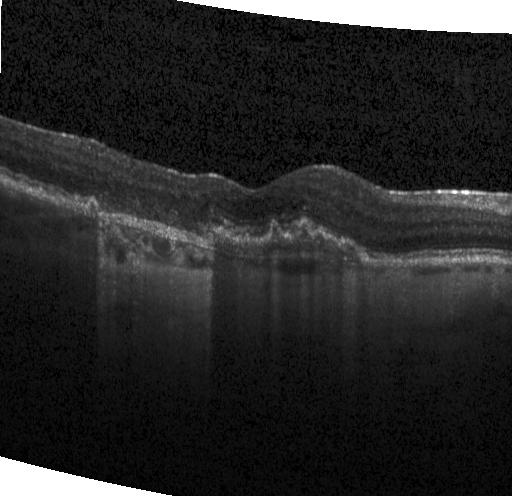 Retinal OCT B-scan · acquired on a Heidelberg Spectralis · fovea-centered — Finding: a choroidal neovascular membrane.